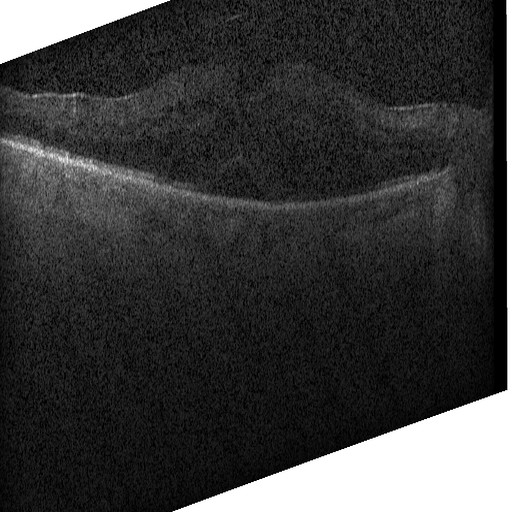

Retinal OCT B-scan; spectral-domain optical coherence tomography — Macular OCT: diabetic macular edema.